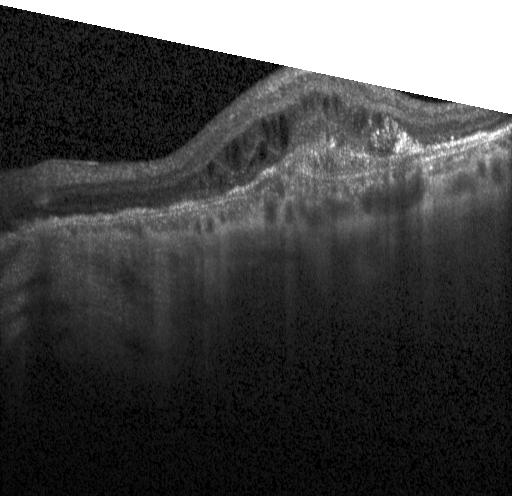 This B-scan demonstrates a choroidal neovascular membrane.